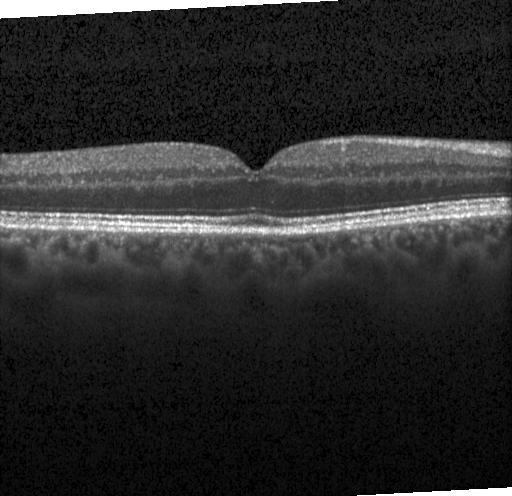
Dx: no choroidal neovascularization, no diabetic macular edema, and no drusen.